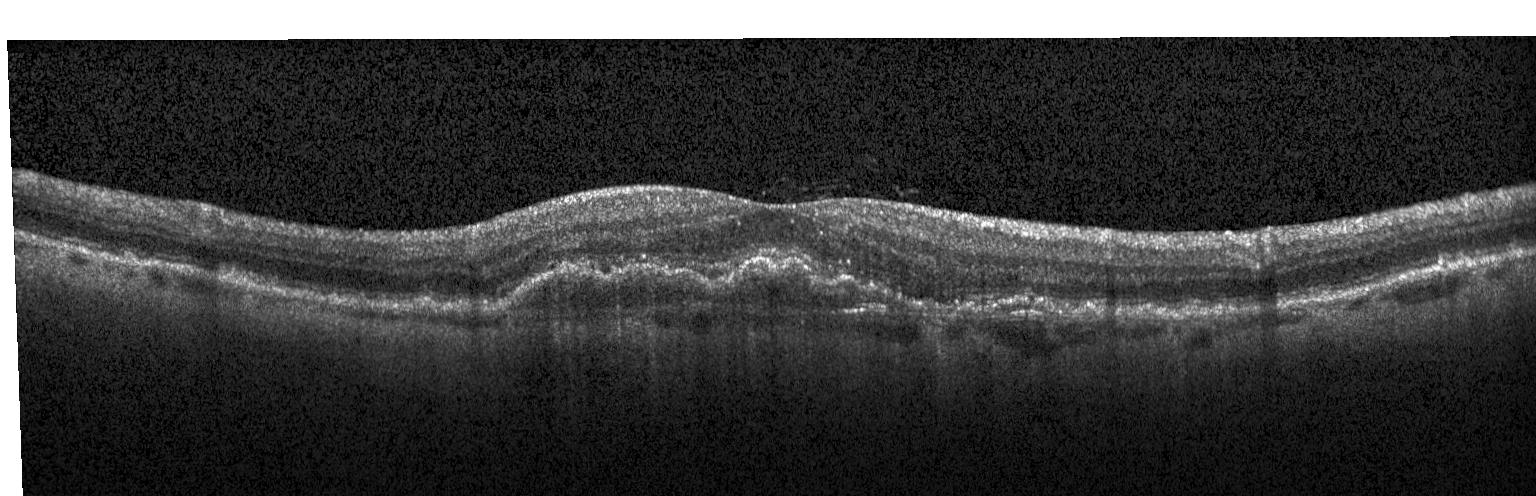

Macular scan · OCT B-scan. Choroidal neovascularization (CNV).